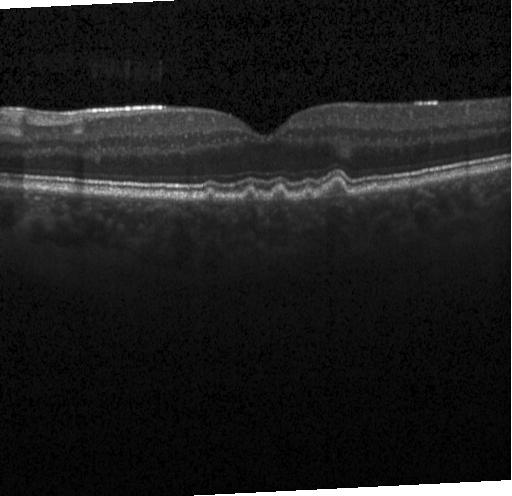
Heidelberg Spectralis · optical coherence tomography B-scan · horizontal scan through the fovea · spectral-domain optical coherence tomography. Dx: sub-RPE drusenoid deposits.